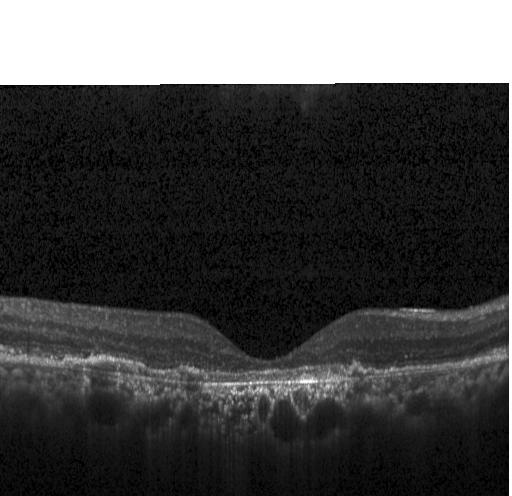 The scan shows choroidal neovascularization (CNV).